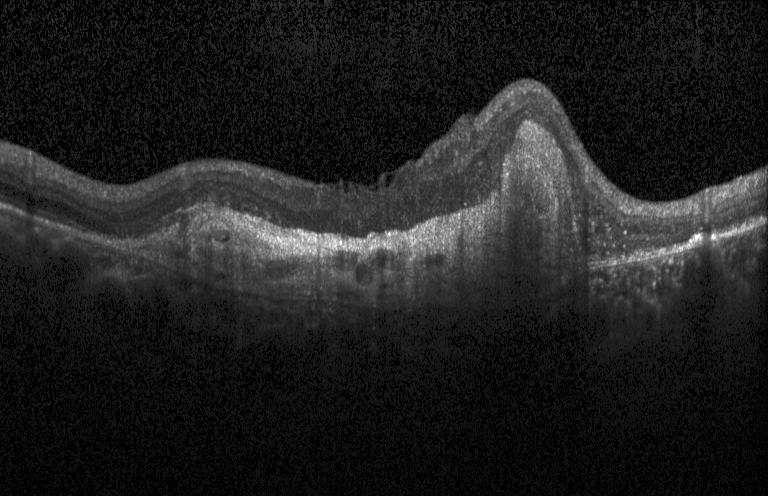 Heidelberg Spectralis, through the macula, retinal OCT B-scan, spectral-domain OCT. CNV.